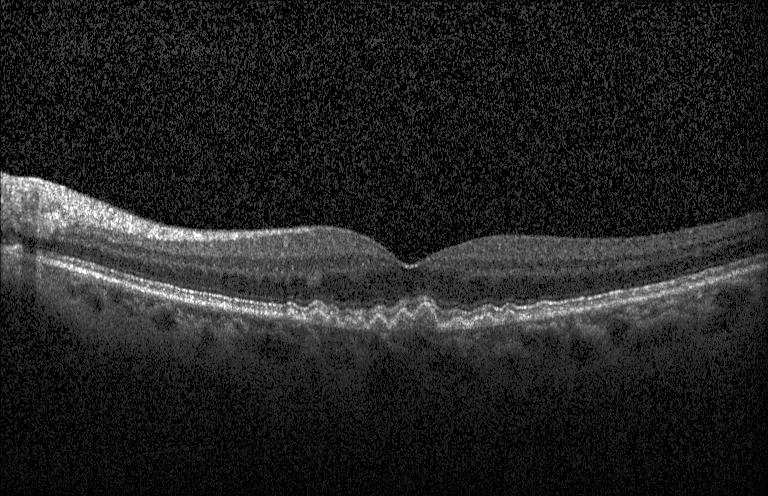
Instrument: Heidelberg Spectralis · spectral-domain OCT · OCT line scan · centered on the fovea.
Finding: sub-RPE drusenoid deposits.